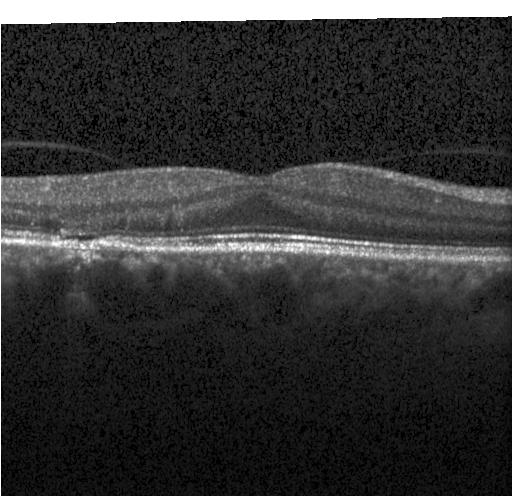 Macular OCT: choroidal neovascularization.